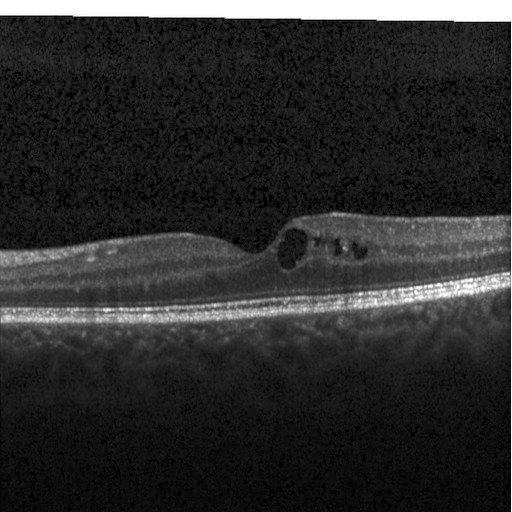 DME.